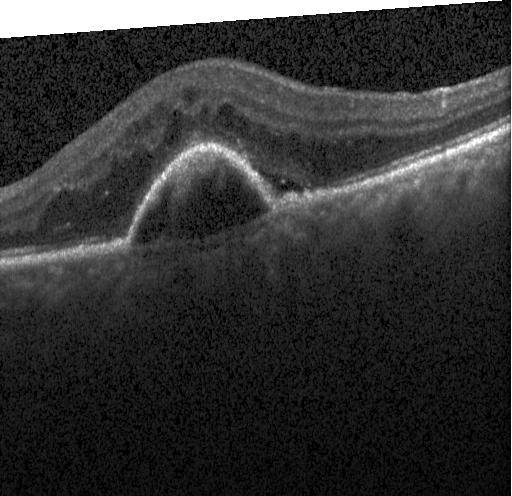 Diagnosis: CNV.